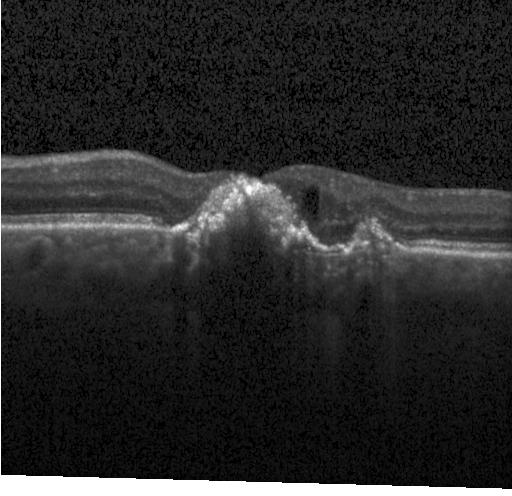
Optical coherence tomography scan. Impression: CNV.